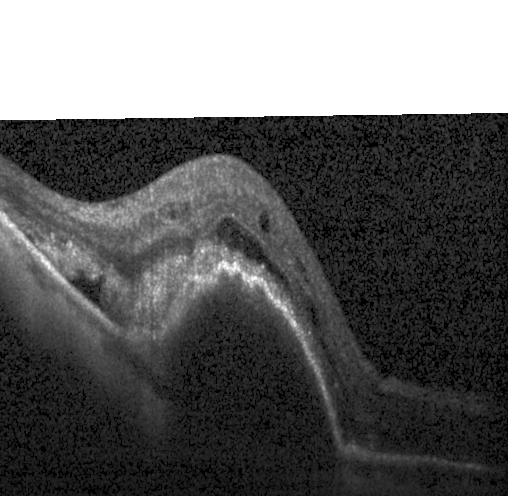 Retinal OCT B-scan · SD-OCT · instrument: Heidelberg Spectralis · centered on the fovea
OCT finding: a choroidal neovascular membrane.